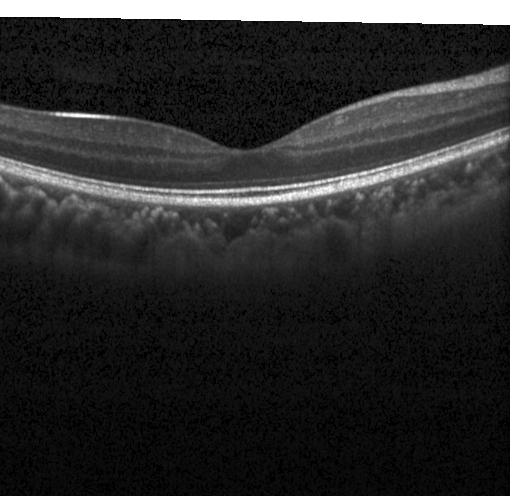 OCT B-scan showing neither CNV, DME, nor drusen.